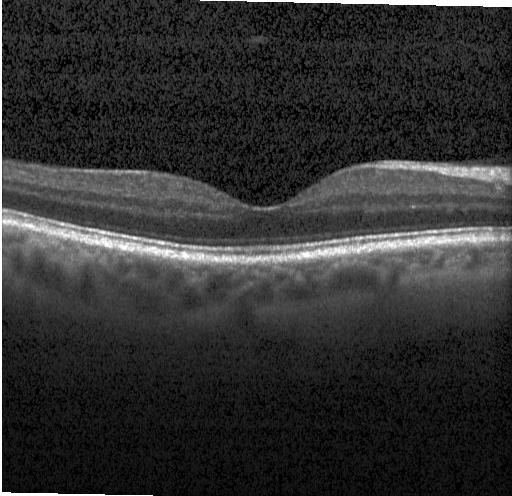

Retinal OCT cross-section. Acquired on a Heidelberg Spectralis. Spectral-domain OCT. Horizontal scan through the fovea
Impression: no CNV, DME, or drusen.